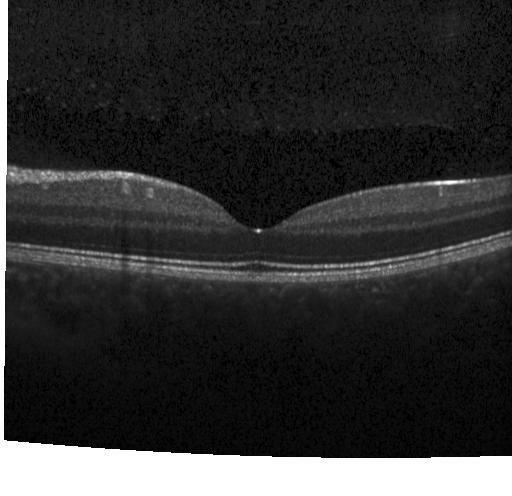 Macular OCT demonstrating neither CNV, DME, nor drusen.